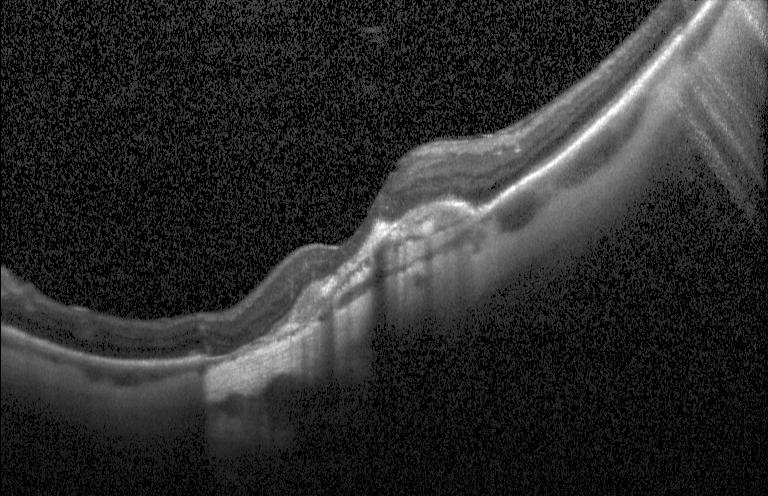
Spectral-domain OCT B-scan: a choroidal neovascular membrane.